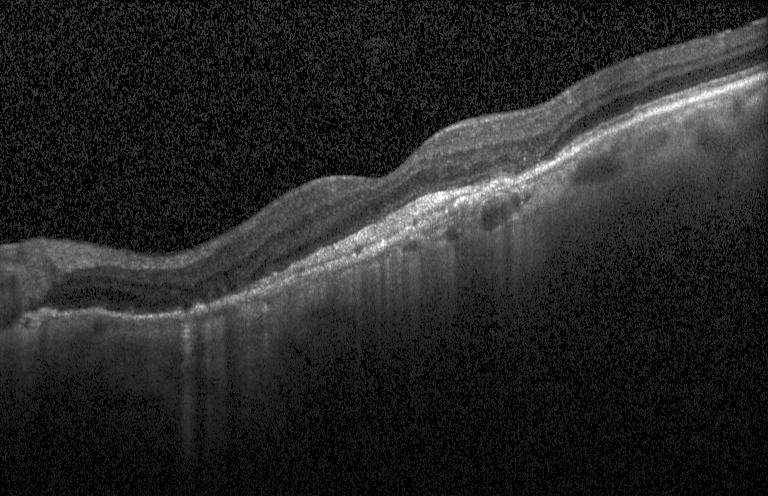
Finding: a choroidal neovascular membrane.